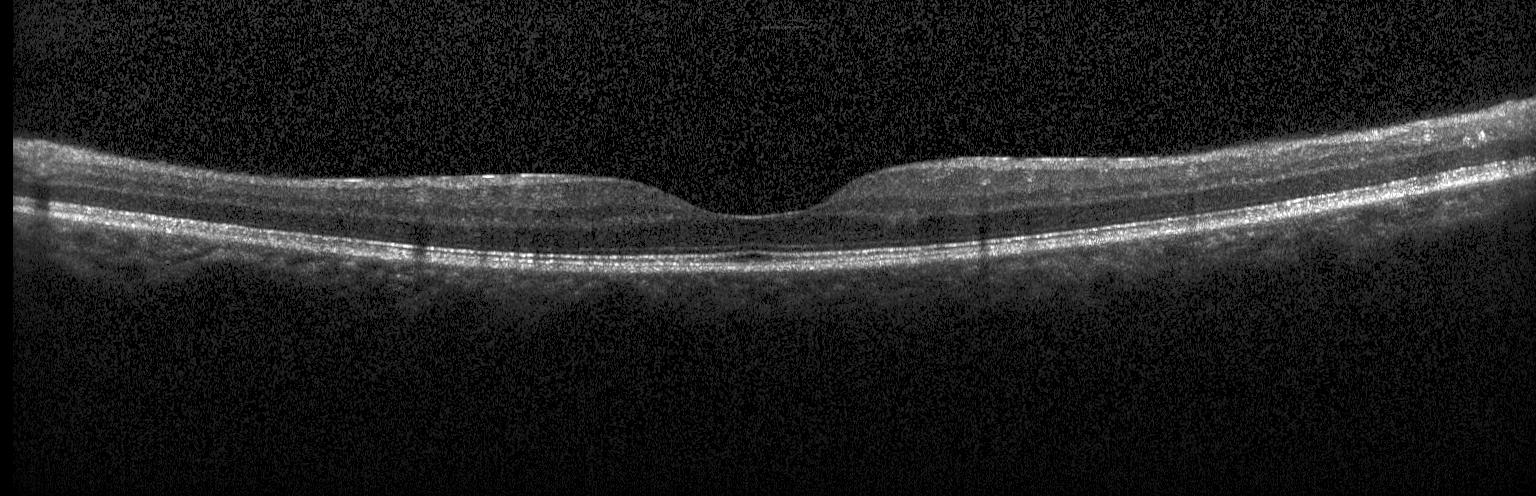 OCT B-scan — Finding: no evidence of choroidal neovascularization, diabetic macular edema, or drusen.